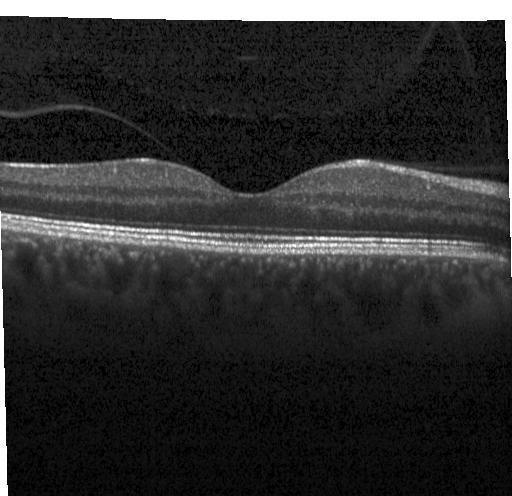
No evidence of choroidal neovascularization, diabetic macular edema, or drusen.